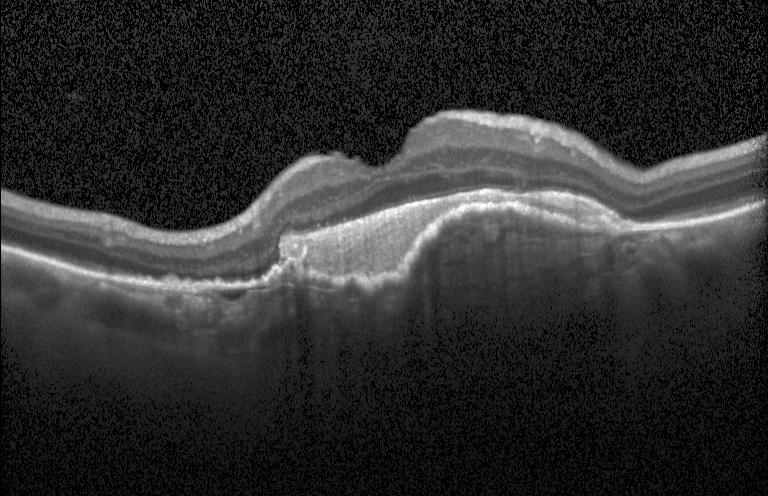

Spectral-domain OCT. Through the macula. Optical coherence tomography B-scan. Instrument: Heidelberg Spectralis
Impression: a choroidal neovascular membrane.